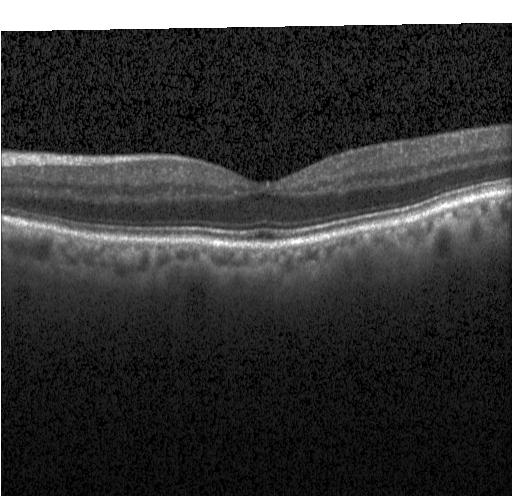 Optical coherence tomography scan. Acquired on a Heidelberg Spectralis. OCT finding: no evidence of CNV, DME, or drusen.